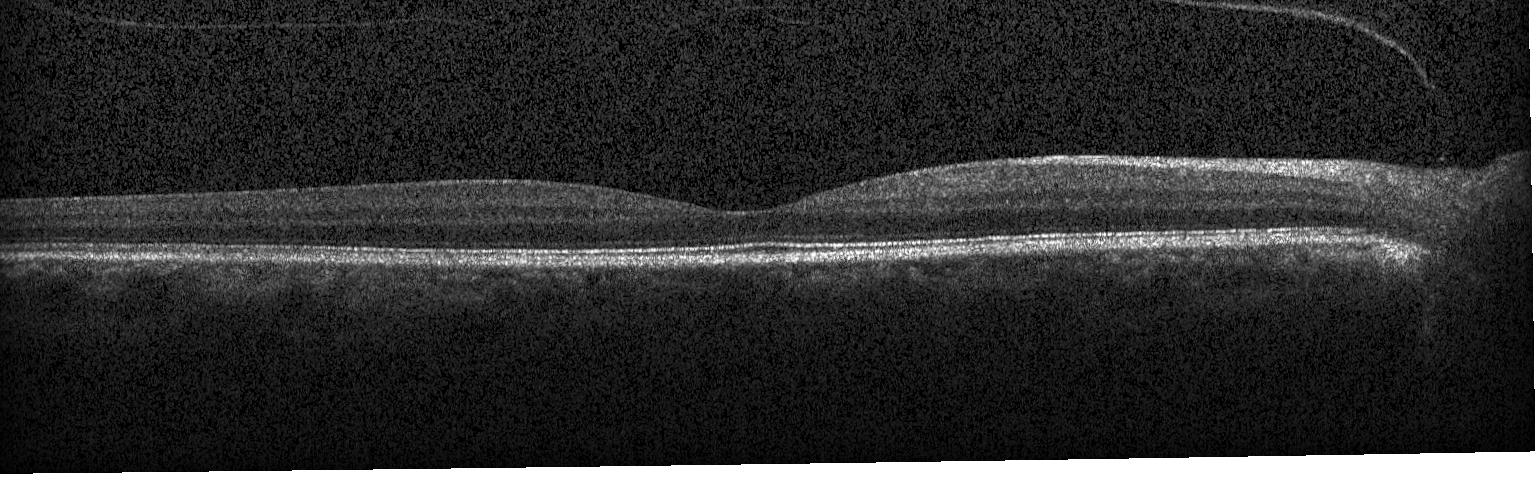

OCT line scan. OCT finding: no choroidal neovascularization, diabetic macular edema, or drusen.